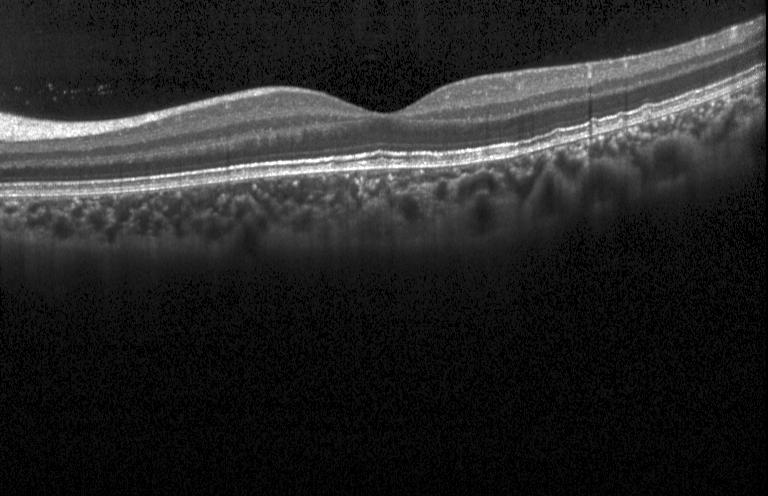
OCT B-scan.
Diagnosis: no CNV, DME, or drusen.